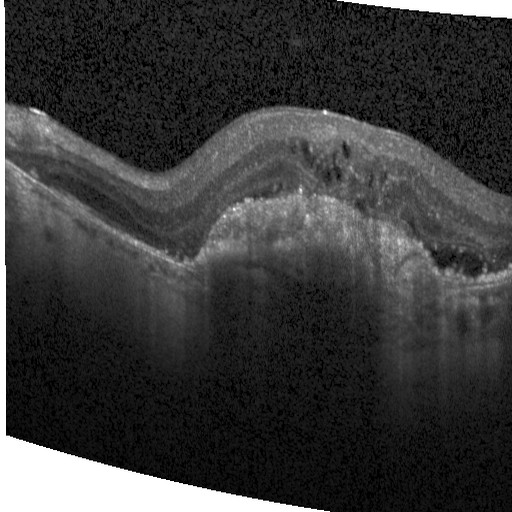
Macular OCT: DME.